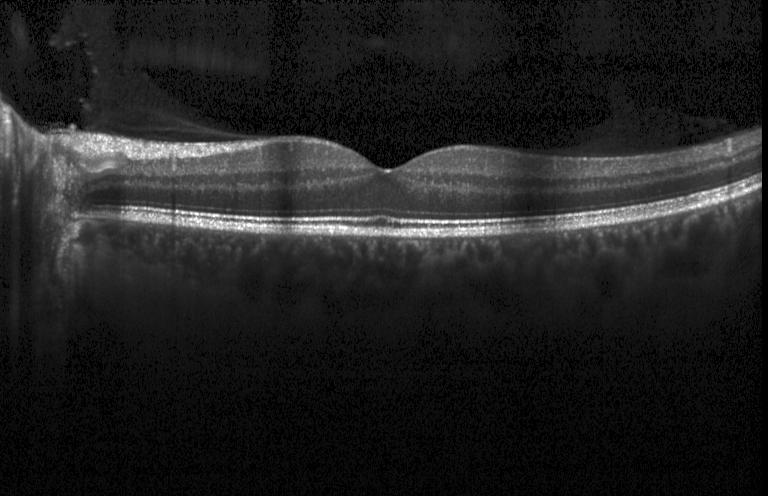
Optical coherence tomography B-scan. Through the macula. Spectral-domain OCT. Acquired on a Heidelberg Spectralis. Macular OCT: no choroidal neovascularization, diabetic macular edema, or drusen.